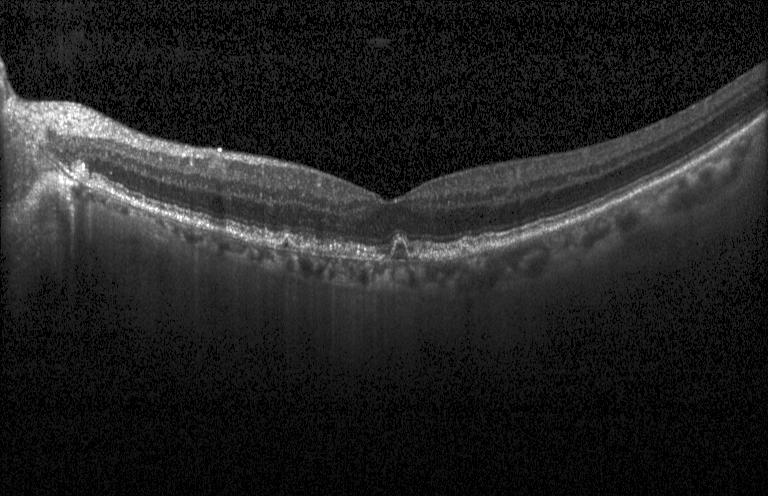 Retinal OCT cross-section — Assessment: sub-RPE drusenoid deposits.